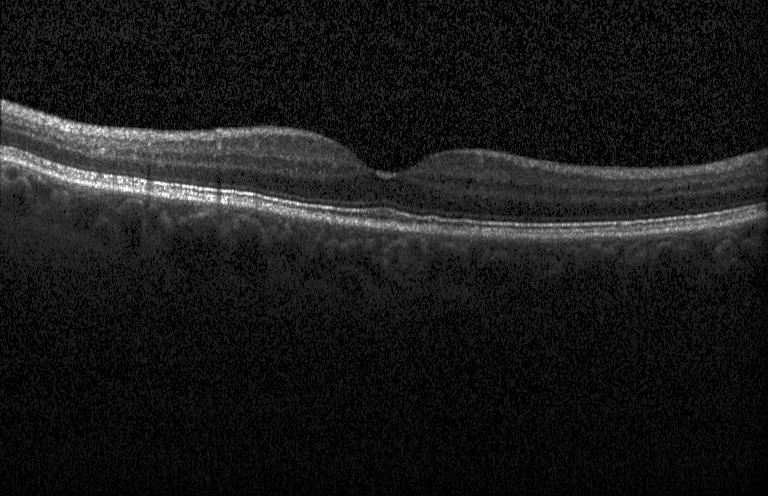
Retinal OCT cross-section; centered on the fovea; instrument: Heidelberg Spectralis; spectral-domain OCT. The scan shows no evidence of CNV, DME, or drusen.